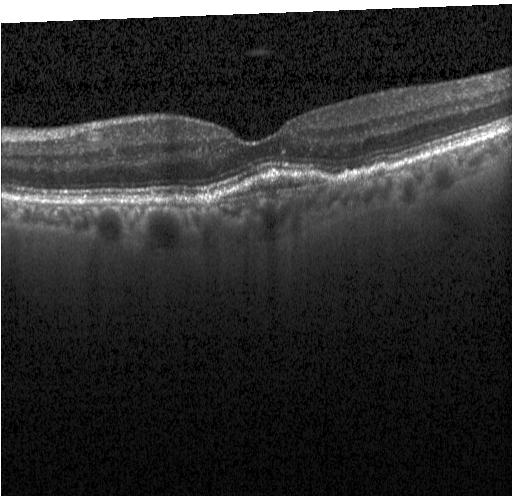

Instrument: Heidelberg Spectralis · fovea-centered · OCT line scan — Finding: choroidal neovascularization.